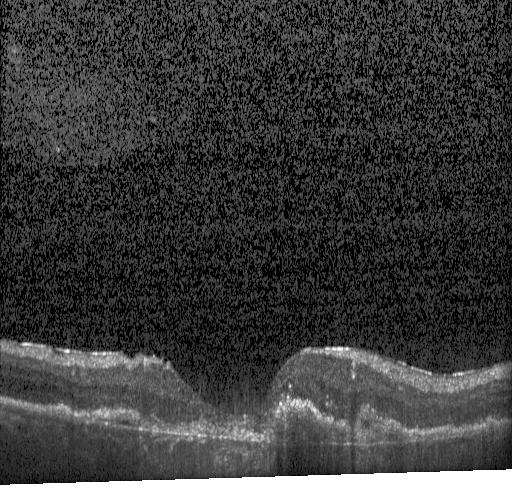 Optical coherence tomography scan — This B-scan demonstrates a choroidal neovascular membrane.